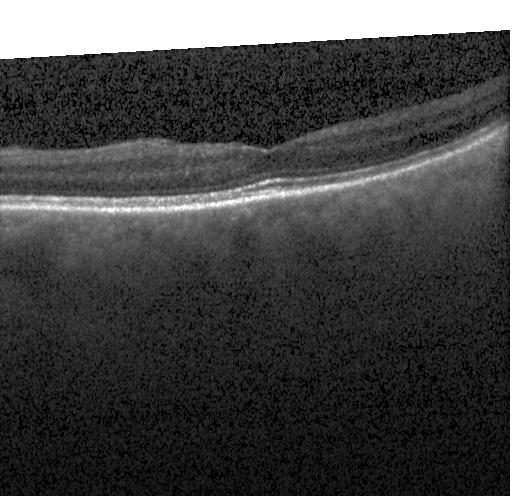 Diagnosis: no evidence of choroidal neovascularization, diabetic macular edema, or drusen.